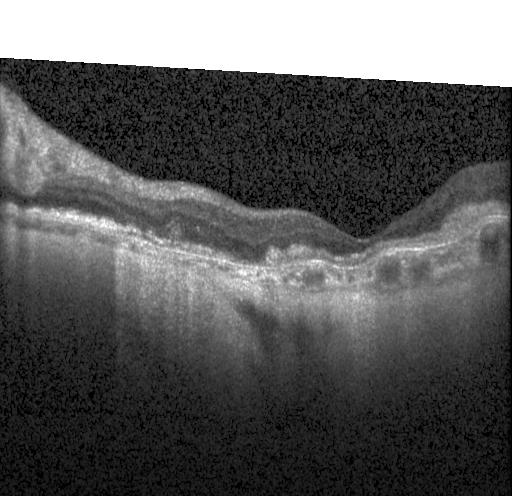
A choroidal neovascular membrane.